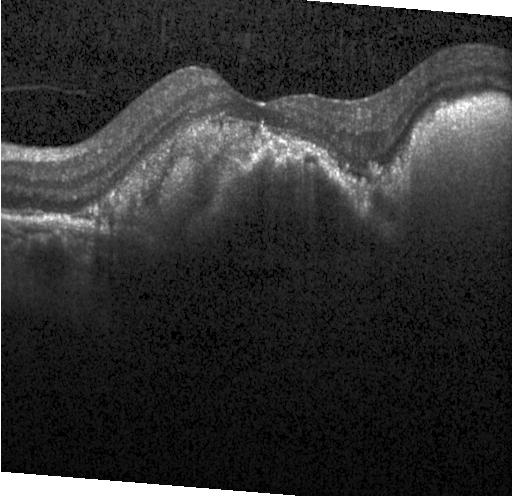 Retinal OCT B-scan. Impression: a choroidal neovascular membrane.